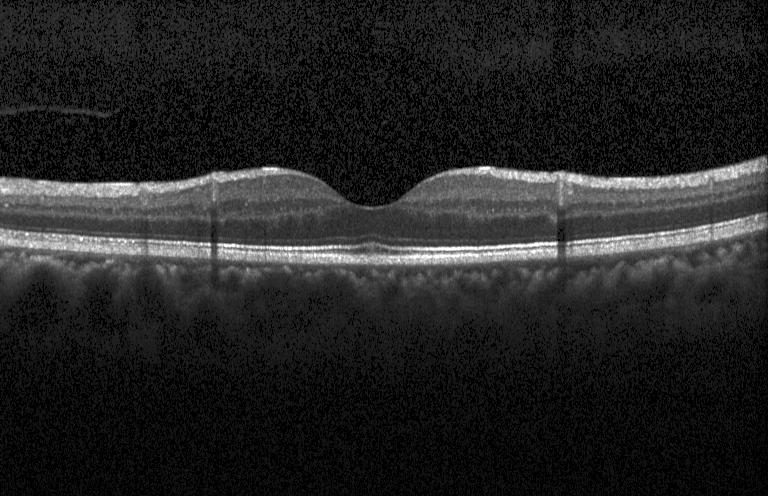

Dx: neither choroidal neovascularization, diabetic macular edema, nor drusen.